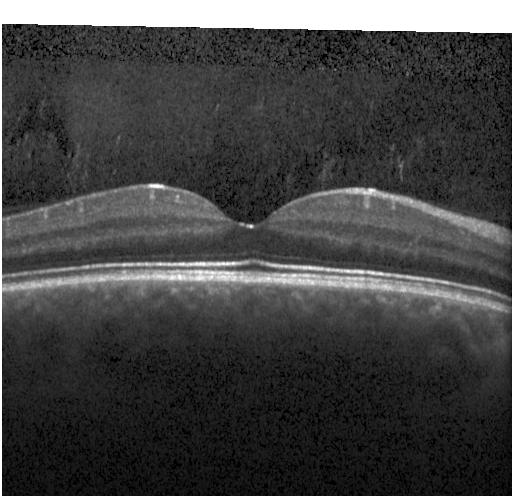

Retinal OCT cross-section, acquired on a Heidelberg Spectralis — Finding: no choroidal neovascularization, no diabetic macular edema, and no drusen.